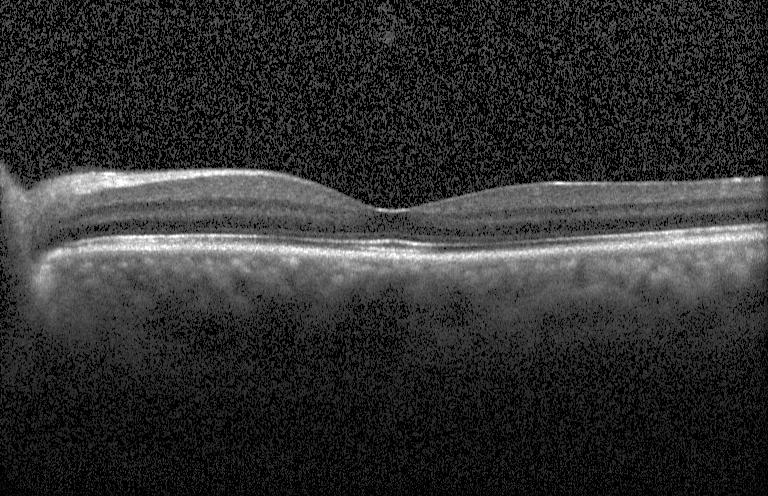
Heidelberg Spectralis. Retinal OCT B-scan — The scan shows neither choroidal neovascularization, diabetic macular edema, nor drusen.